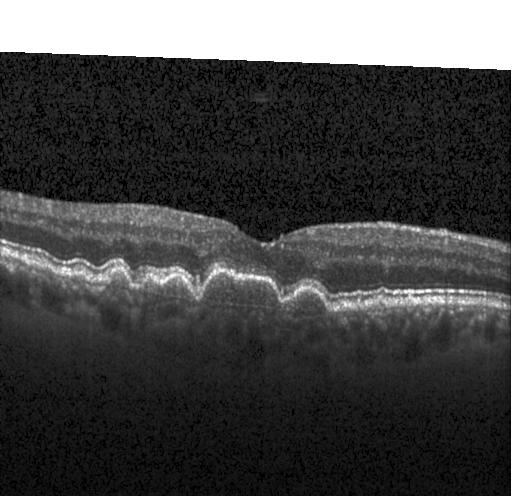
Retinal OCT cross-section, horizontal scan through the fovea, SD-OCT, Heidelberg Spectralis. OCT finding: sub-RPE drusenoid deposits.